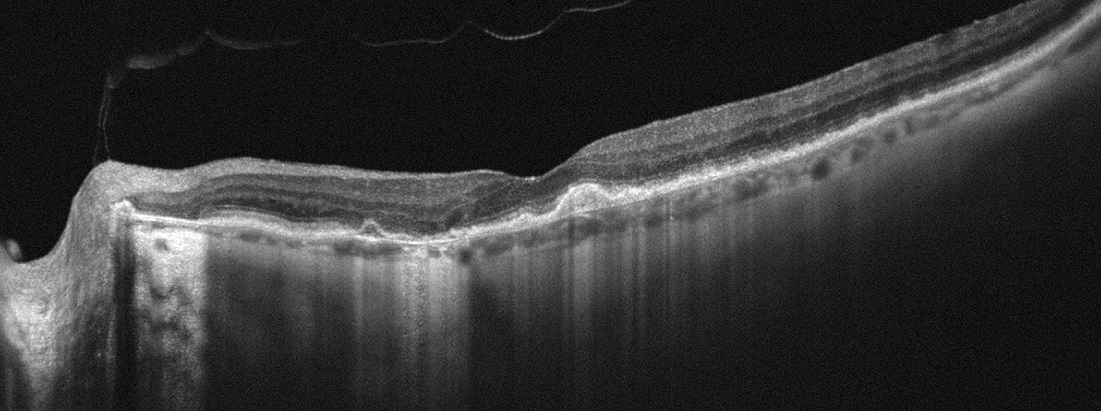
OCT B-scan. Macular scan. Optovue Avanti RTVue XR. Dx: AMD.